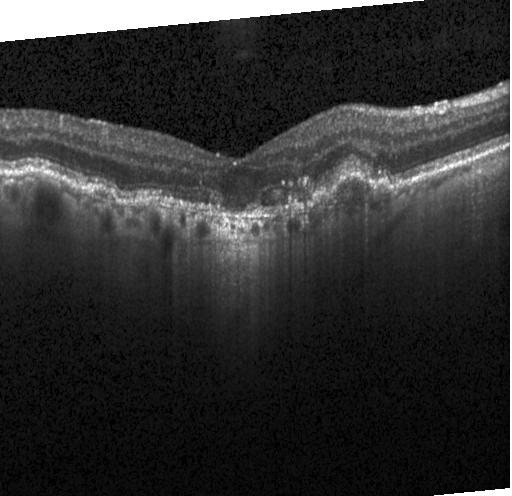
Retinal OCT cross-section
The scan shows choroidal neovascularization (CNV).